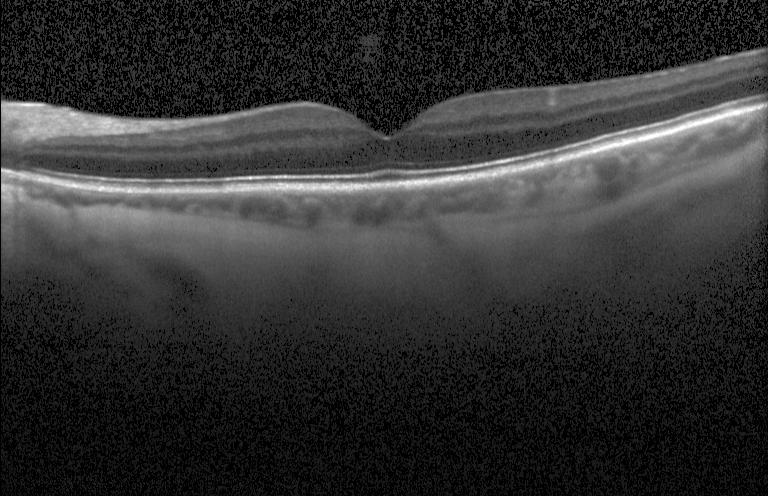

Finding: neither CNV, DME, nor drusen.